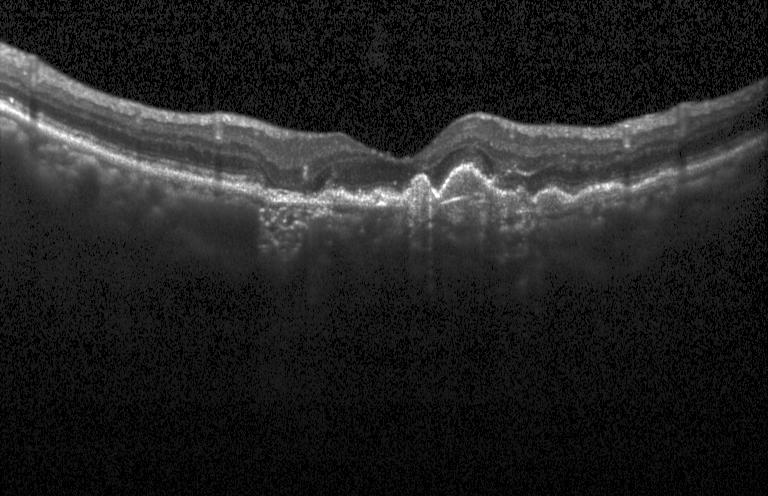
Spectral-domain OCT · OCT line scan
Diagnosis: a choroidal neovascular membrane.